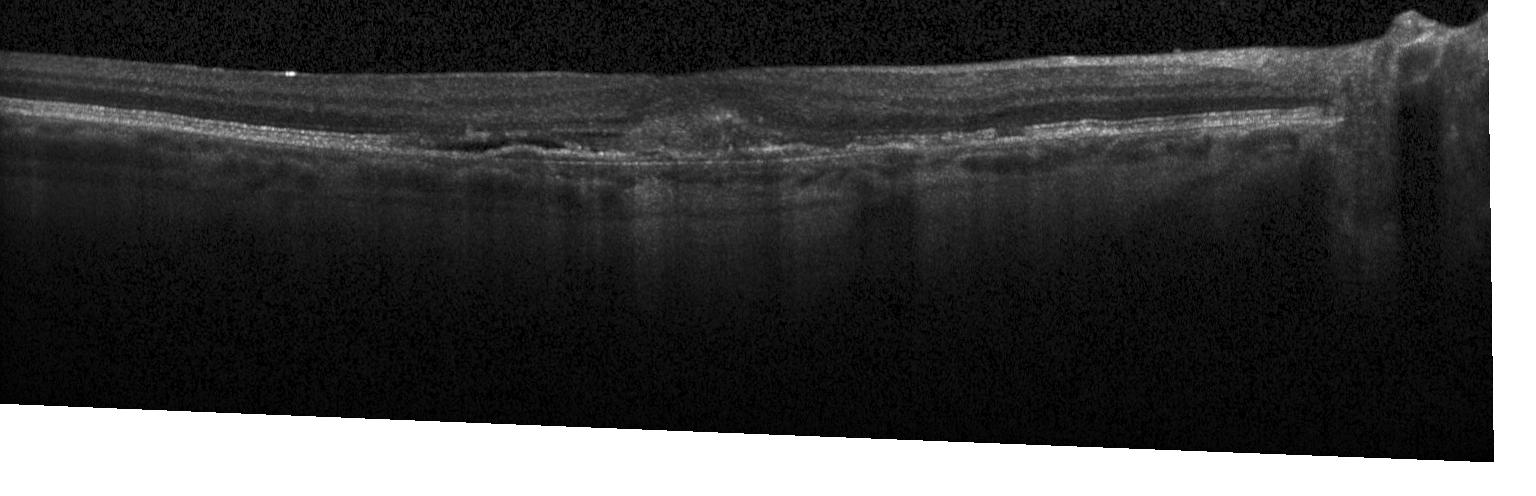 Macular OCT: choroidal neovascularization (CNV).